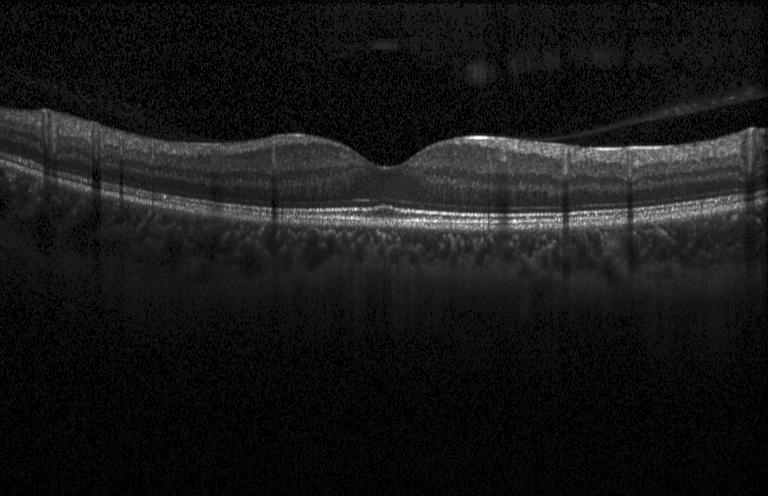

Retinal OCT B-scan · instrument: Heidelberg Spectralis · SD-OCT · fovea-centered — Assessment: no choroidal neovascularization, diabetic macular edema, or drusen.